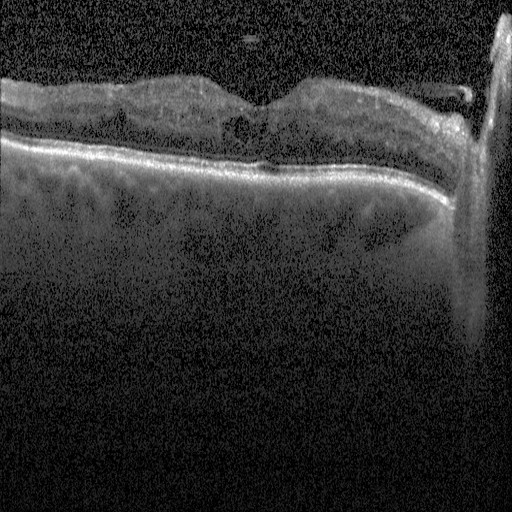 OCT finding: DME.